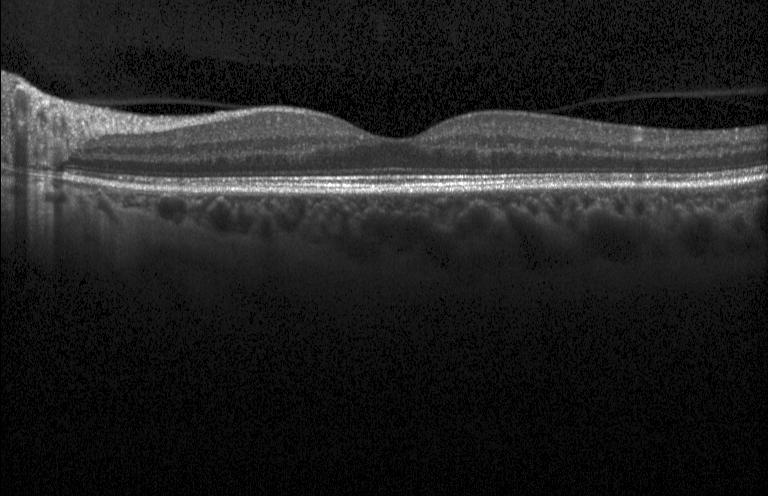
Horizontal scan through the fovea · OCT line scan
Finding: no CNV, no DME, and no drusen.